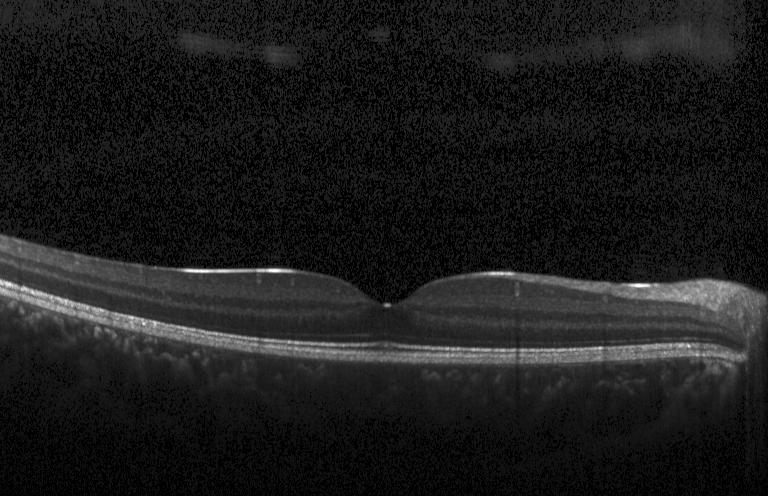
Finding: no choroidal neovascularization, no diabetic macular edema, and no drusen.